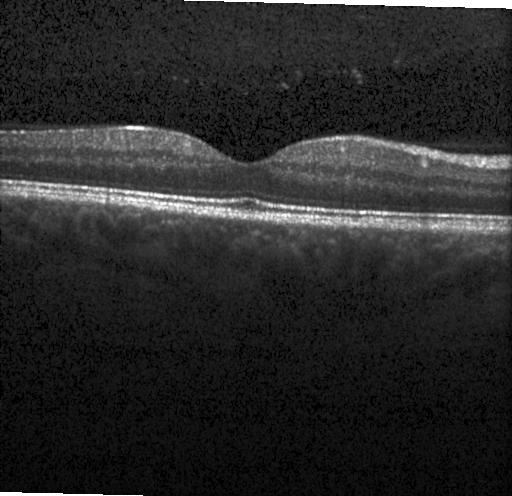
OCT finding: neither choroidal neovascularization, diabetic macular edema, nor drusen.